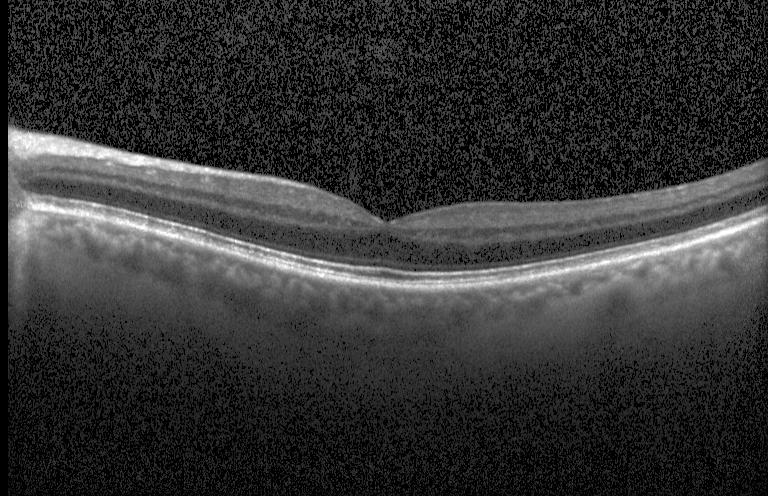

Impression: neither choroidal neovascularization, diabetic macular edema, nor drusen.